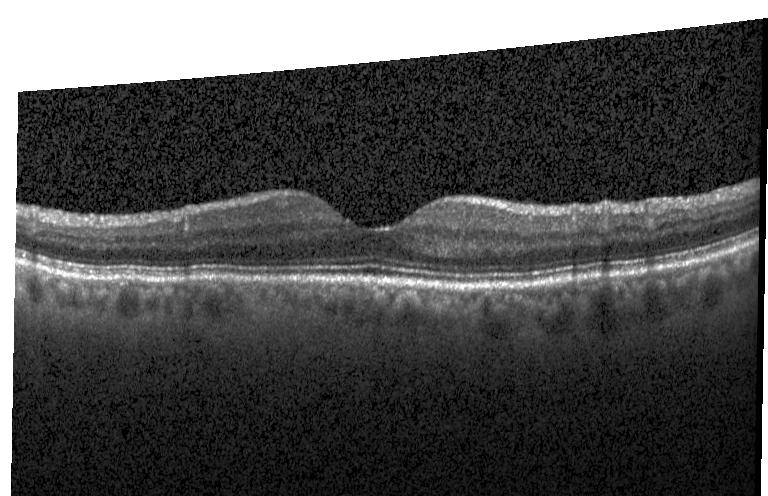
Heidelberg Spectralis OCT system · retinal OCT cross-section · through the macula — OCT finding: no evidence of choroidal neovascularization, diabetic macular edema, or drusen.